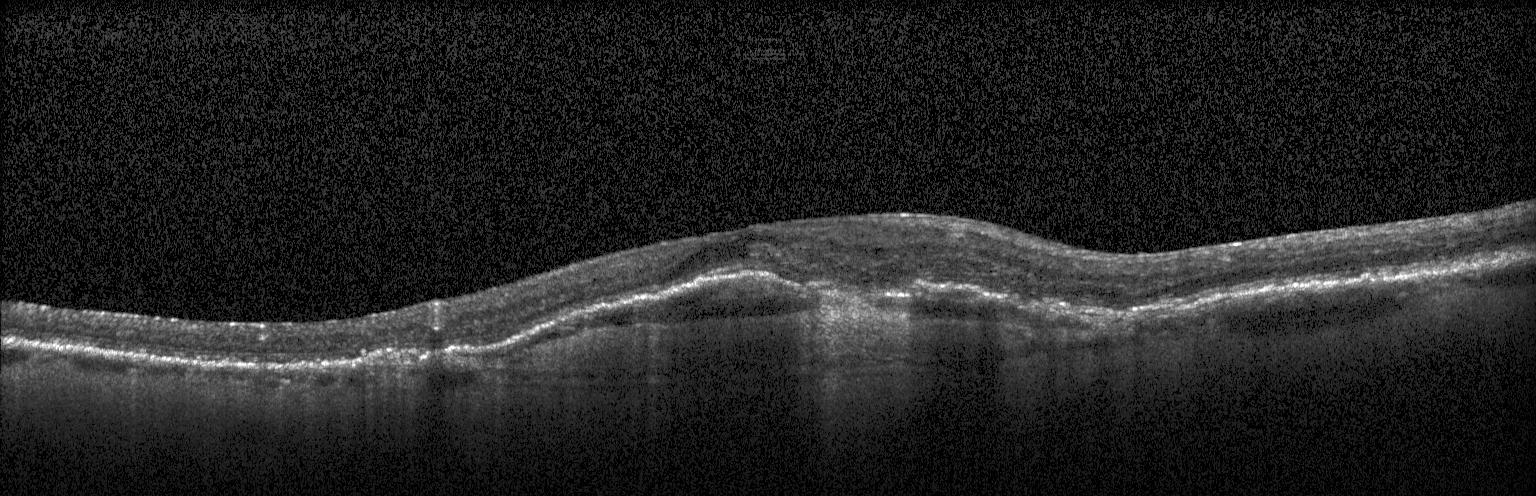 Spectral-domain optical coherence tomography. OCT line scan. Heidelberg Spectralis OCT system. Macular scan
OCT finding: choroidal neovascularization (CNV).